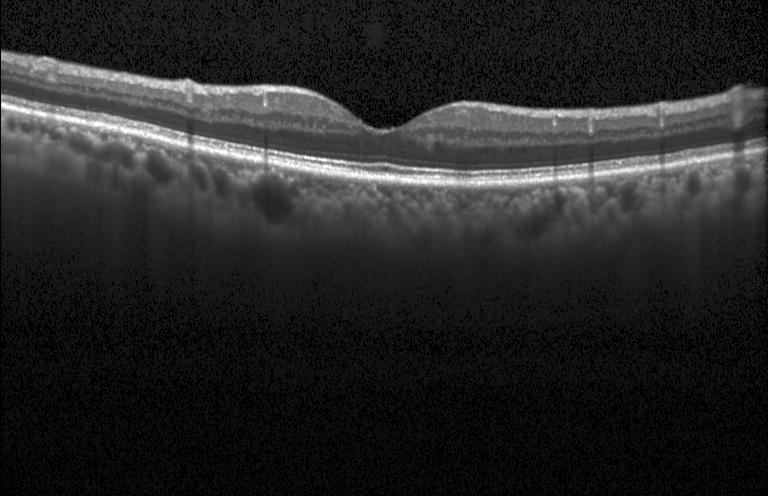 Finding: no evidence of choroidal neovascularization, diabetic macular edema, or drusen.